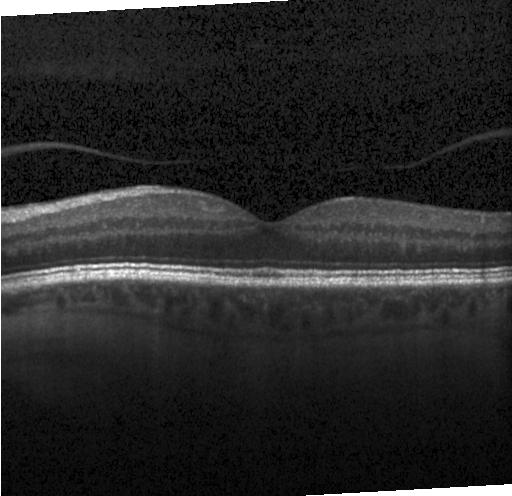
The scan shows no choroidal neovascularization, diabetic macular edema, or drusen.